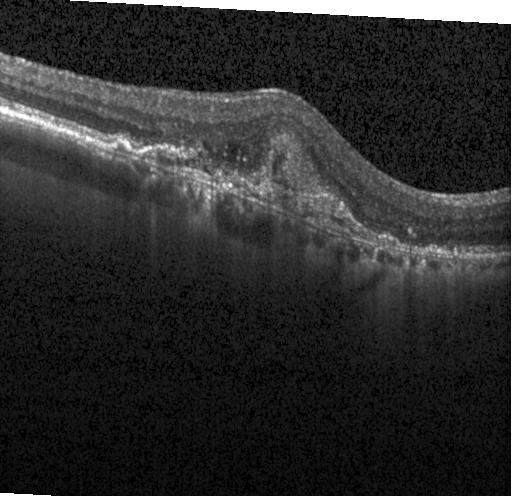 OCT scan showing a choroidal neovascular membrane.